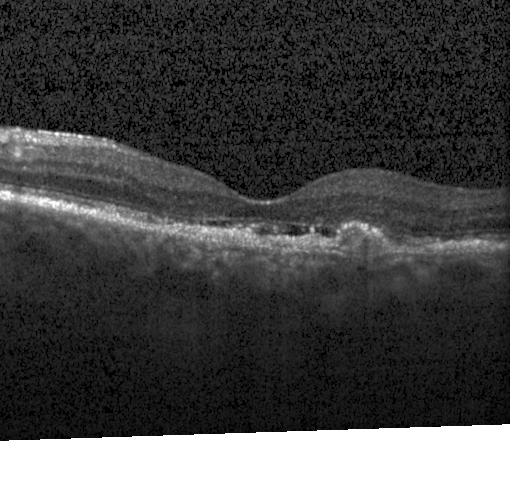

Acquired on a Heidelberg Spectralis; spectral-domain OCT; retinal OCT cross-section; centered on the fovea. This B-scan demonstrates CNV.